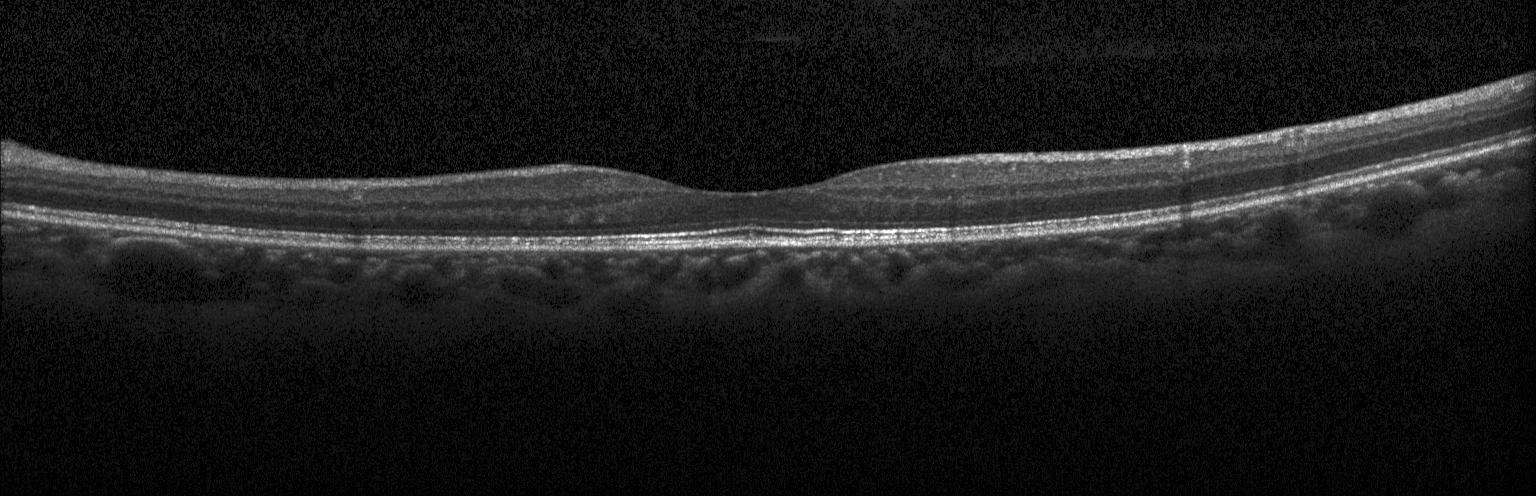
Fovea-centered. SD-OCT. Optical coherence tomography B-scan
Finding: no choroidal neovascularization, diabetic macular edema, or drusen.